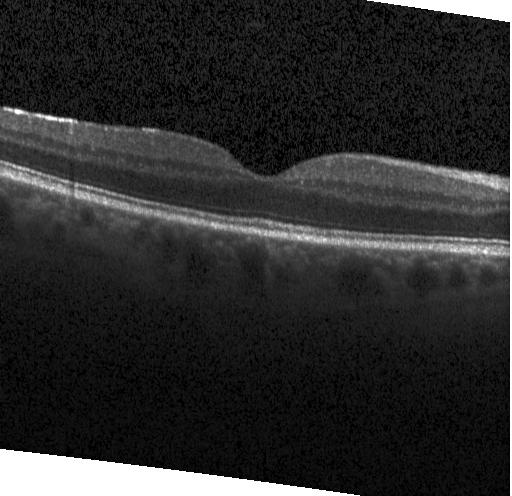
Heidelberg Spectralis · retinal OCT B-scan — Diagnosis: no choroidal neovascularization, diabetic macular edema, or drusen.